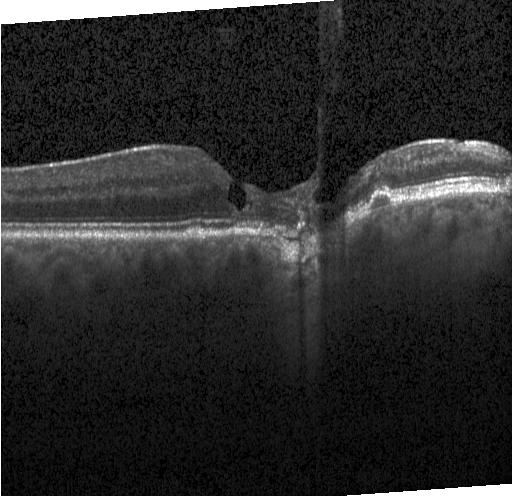 Optical coherence tomography B-scan. Heidelberg Spectralis — The scan shows CNV.